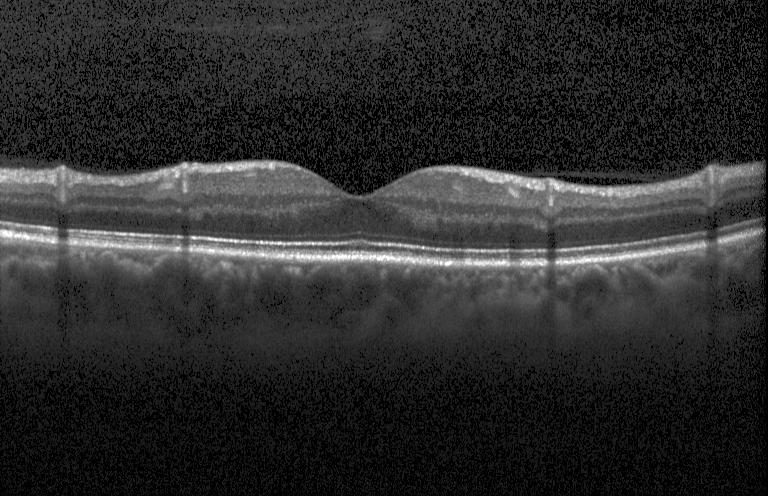 Macular scan, instrument: Heidelberg Spectralis, spectral-domain OCT, optical coherence tomography B-scan. Macular OCT: no choroidal neovascularization, no diabetic macular edema, and no drusen.